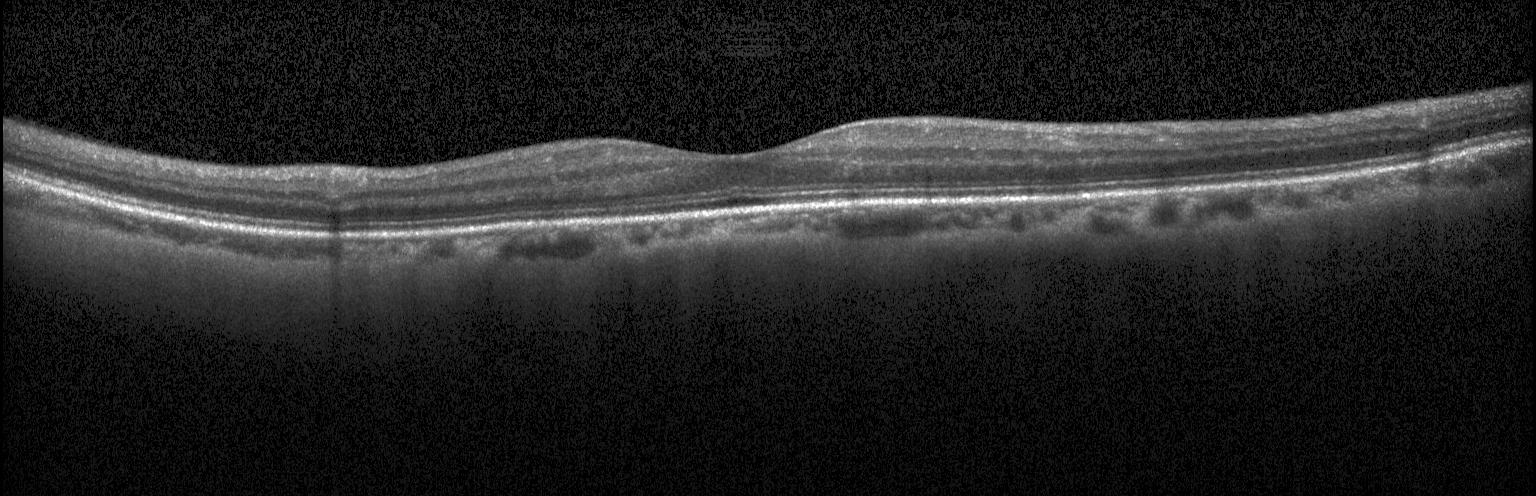
The scan shows no choroidal neovascularization, diabetic macular edema, or drusen.